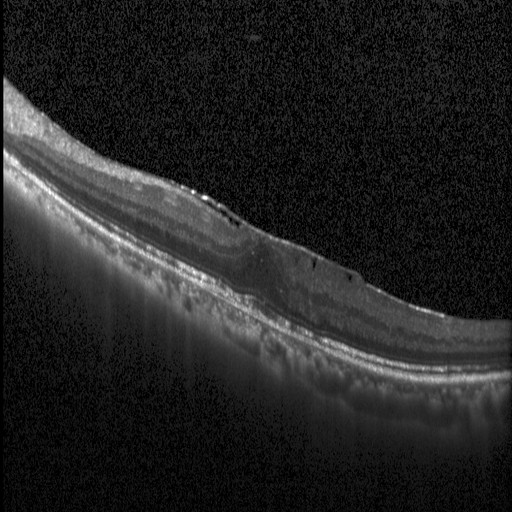
Optical coherence tomography B-scan · horizontal scan through the fovea · spectral-domain optical coherence tomography · Heidelberg Spectralis OCT system.
Diagnosis: diabetic macular edema.